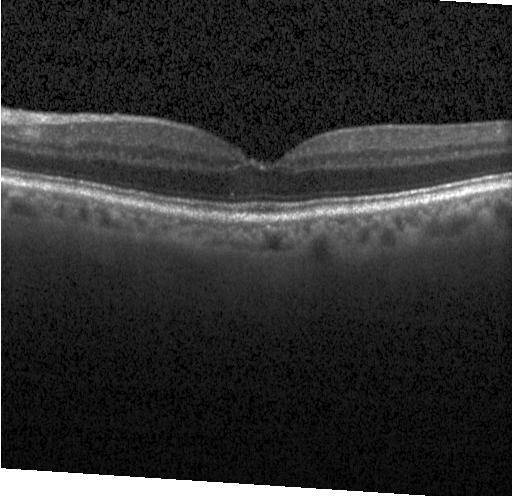
Optical coherence tomography scan · SD-OCT · macular scan · acquired on a Heidelberg Spectralis
The scan shows no CNV, no DME, and no drusen.